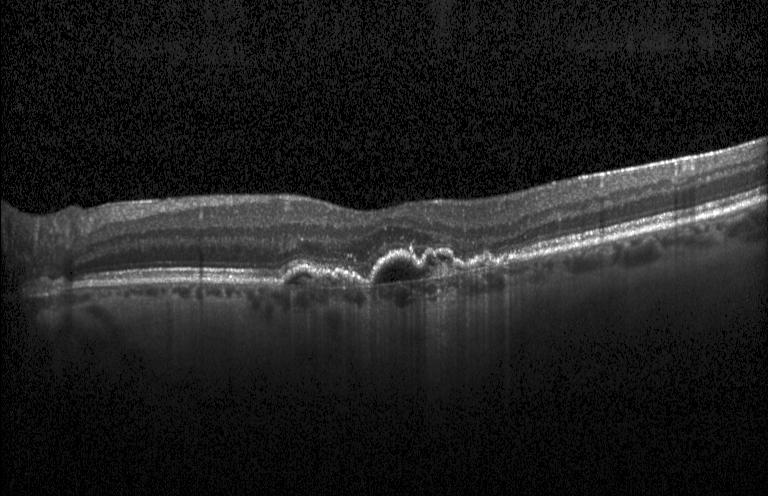

Spectral-domain optical coherence tomography, horizontal scan through the fovea, optical coherence tomography B-scan — Dx: CNV.